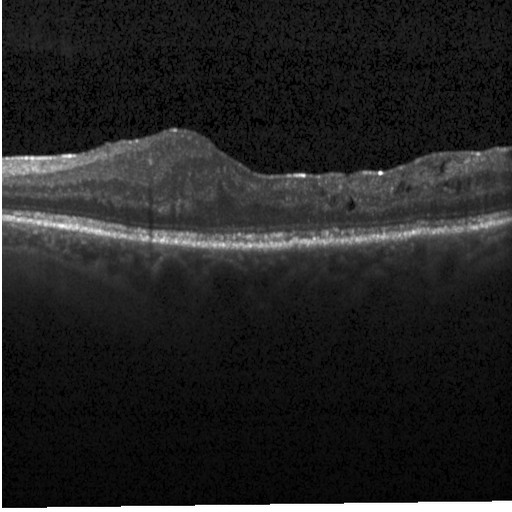
Optical coherence tomography B-scan — Finding: diabetic macular edema (DME).